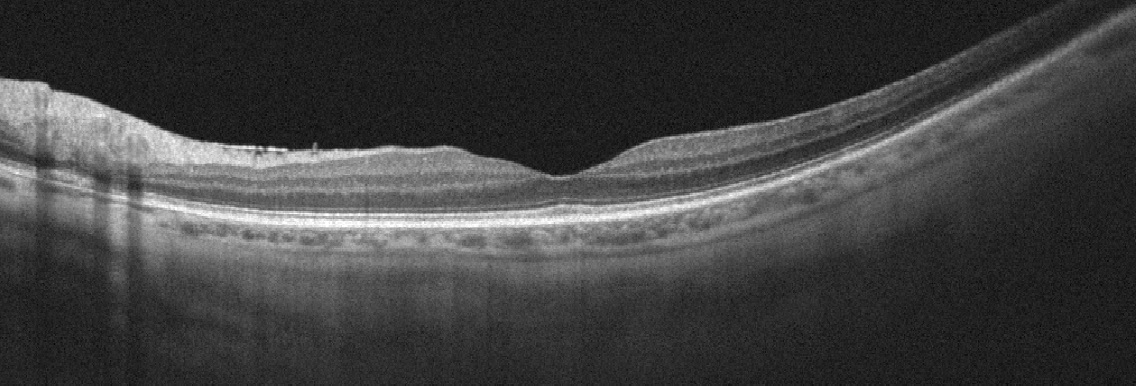 Diagnosis: epiretinal membrane.